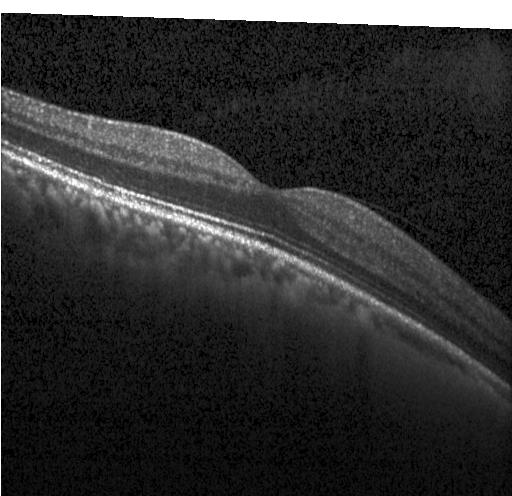

Heidelberg Spectralis OCT system. OCT B-scan. Spectral-domain OCT. Macular scan — This B-scan demonstrates neither CNV, DME, nor drusen.